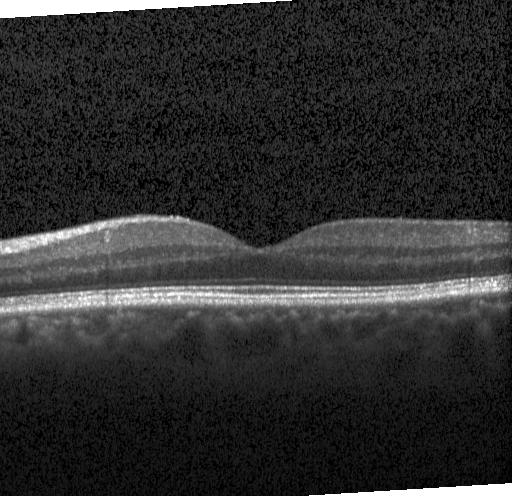

Impression: no choroidal neovascularization, no diabetic macular edema, and no drusen.